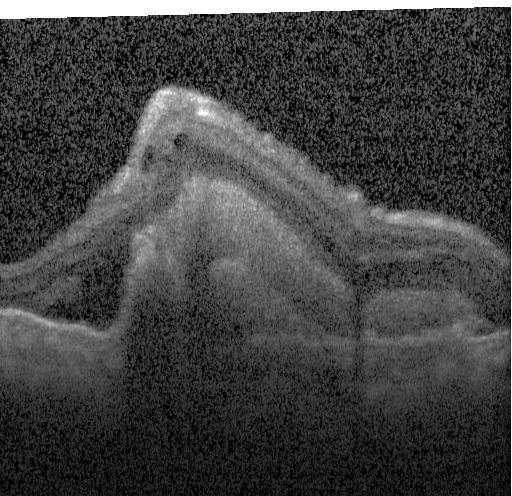 OCT B-scan.
Assessment: a choroidal neovascular membrane.